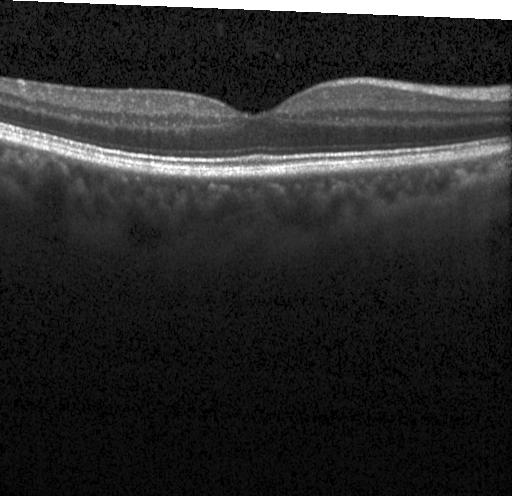
OCT finding: neither CNV, DME, nor drusen.